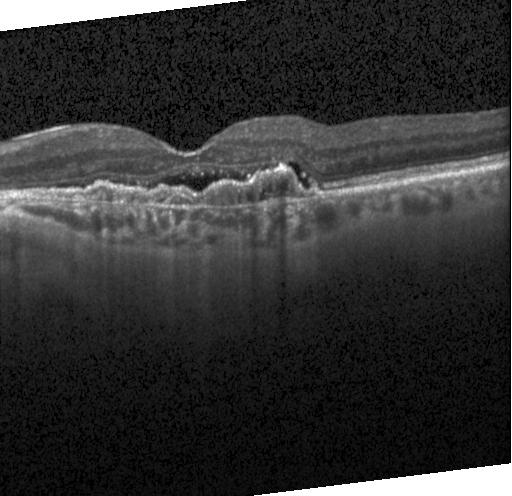
Macular OCT: choroidal neovascularization.